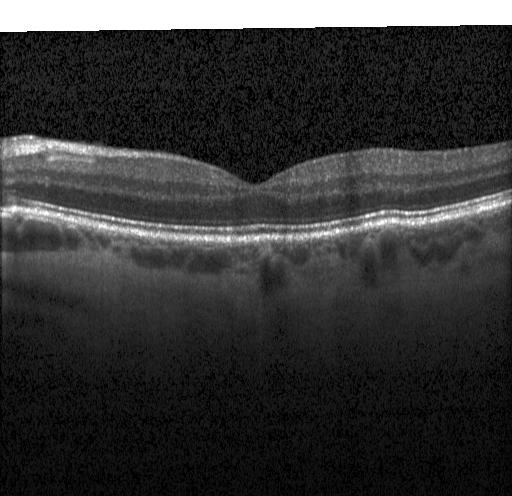 Acquired on a Heidelberg Spectralis · retinal OCT cross-section
Assessment: neither choroidal neovascularization, diabetic macular edema, nor drusen.